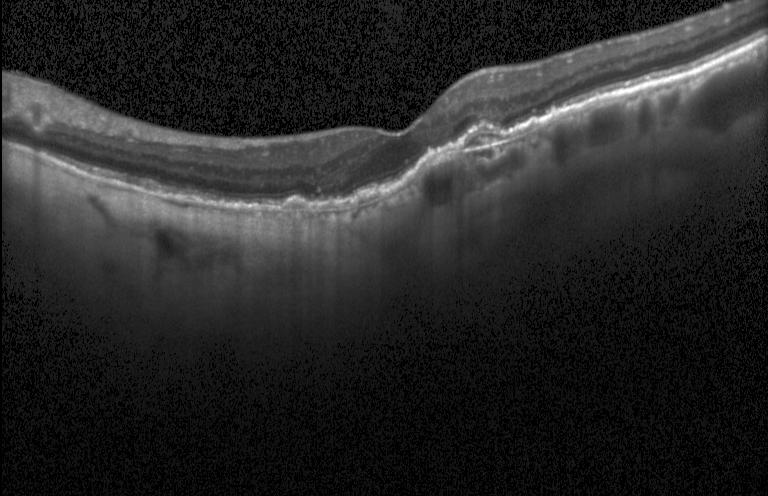
Diagnosis: a choroidal neovascular membrane.